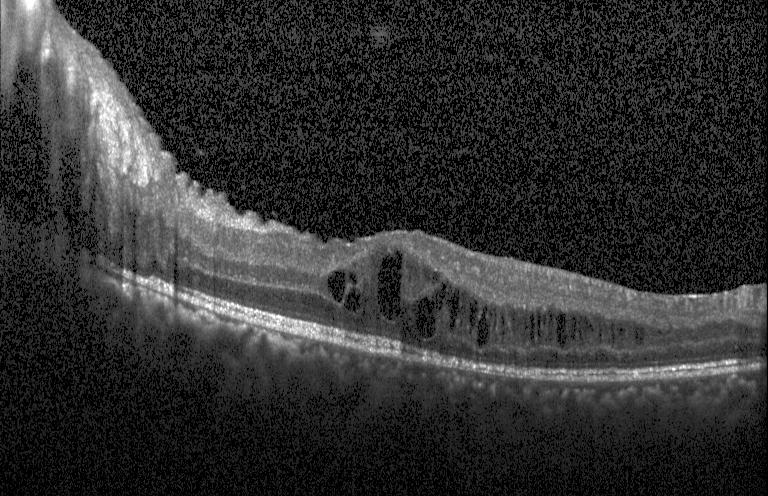

Macular scan · instrument: Heidelberg Spectralis · optical coherence tomography scan. Diagnosis: diabetic macular edema (DME).